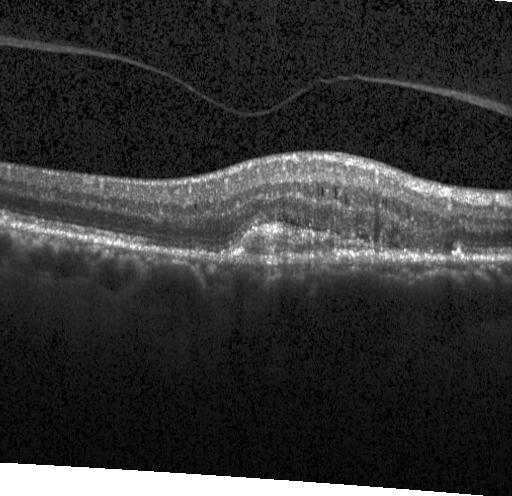
Heidelberg Spectralis OCT system; retinal OCT cross-section — Macular OCT: choroidal neovascularization.